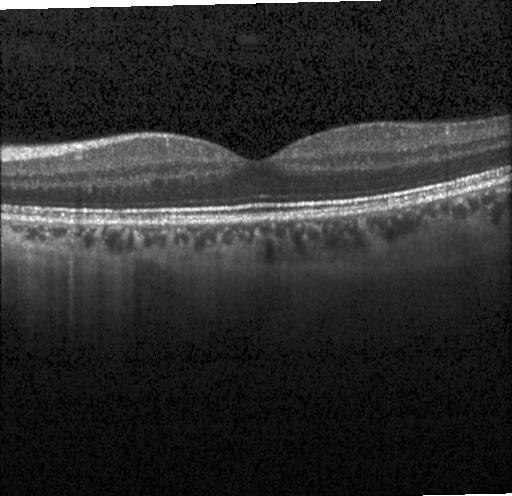

Spectral-domain OCT; Heidelberg Spectralis; retinal OCT B-scan; horizontal scan through the fovea — Diagnosis: no evidence of choroidal neovascularization, diabetic macular edema, or drusen.